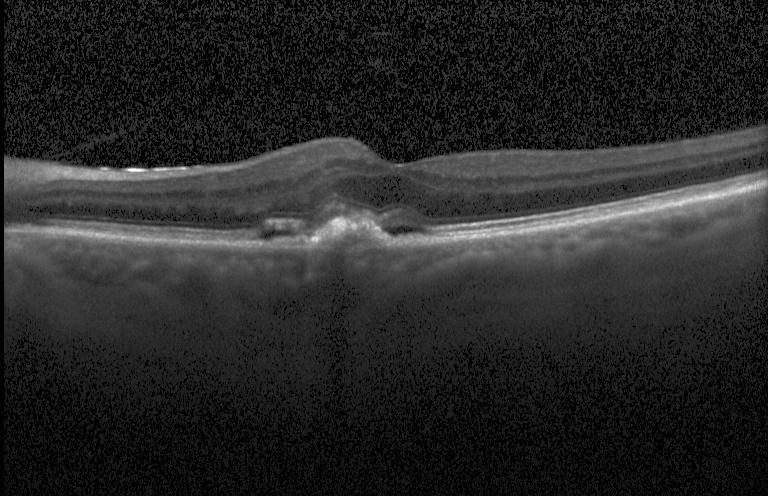

Macular OCT: choroidal neovascularization (CNV).